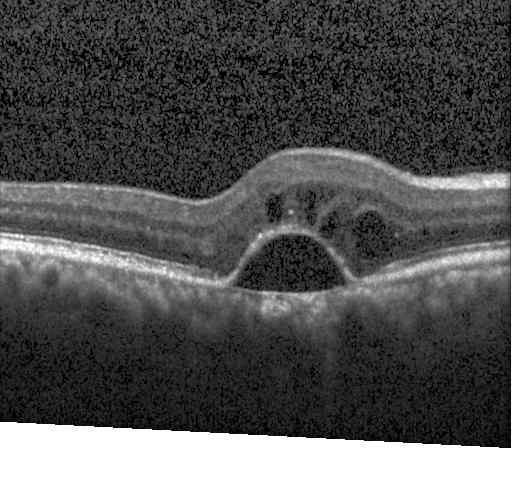
Spectral-domain OCT. Instrument: Heidelberg Spectralis. Retinal OCT cross-section. Impression: a choroidal neovascular membrane.